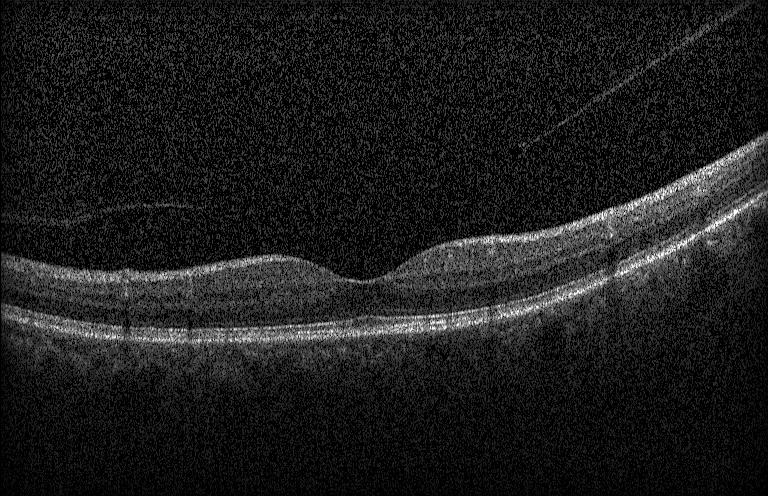 OCT scan showing no choroidal neovascularization, no diabetic macular edema, and no drusen.